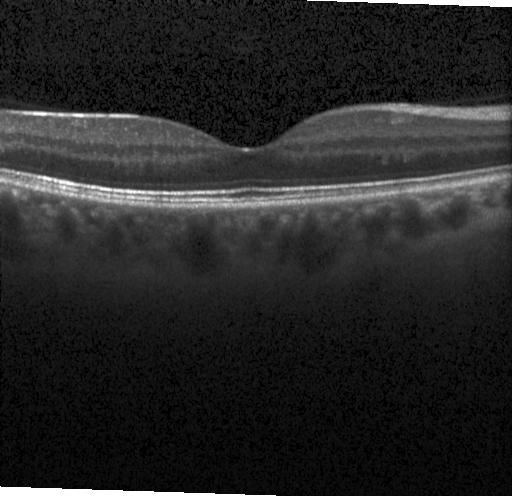
Optical coherence tomography scan
Impression: no evidence of choroidal neovascularization, diabetic macular edema, or drusen.